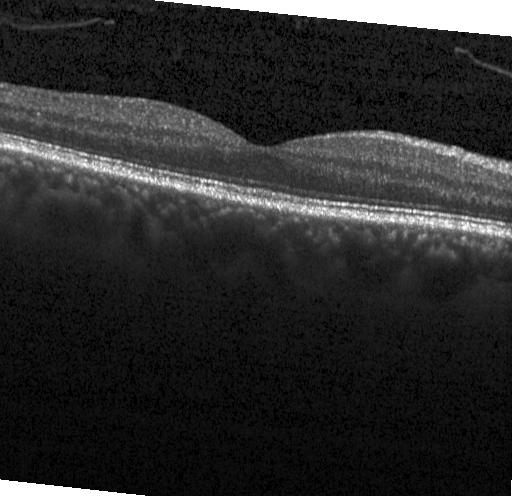
Optical coherence tomography scan · spectral-domain optical coherence tomography — OCT finding: no evidence of CNV, DME, or drusen.